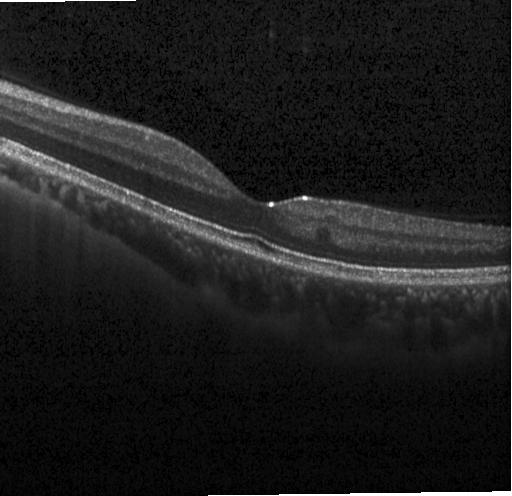

Spectral-domain OCT · instrument: Heidelberg Spectralis · optical coherence tomography B-scan — Impression: no choroidal neovascularization, diabetic macular edema, or drusen.